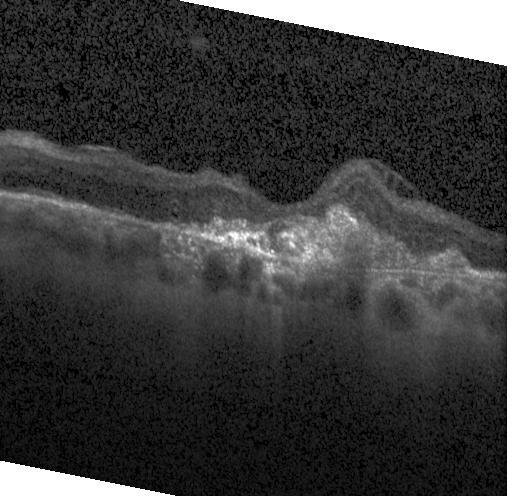
Retinal OCT cross-section showing choroidal neovascularization (CNV).